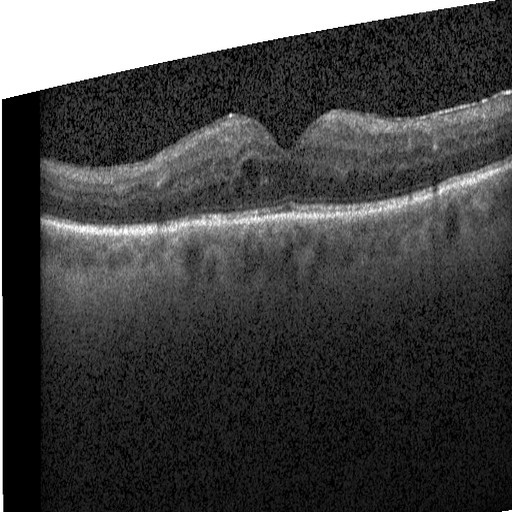 Through the macula; SD-OCT; optical coherence tomography scan — OCT finding: diabetic macular edema.